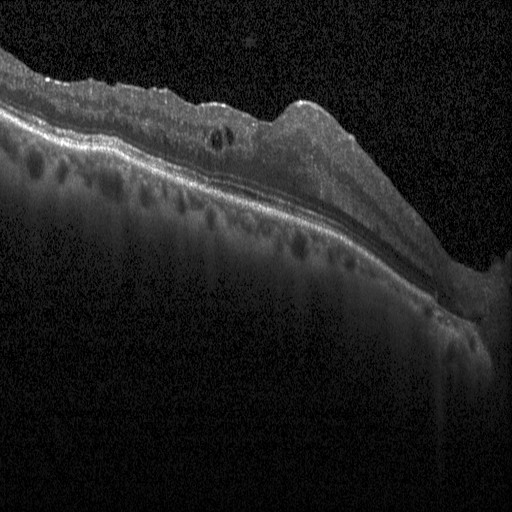
This B-scan demonstrates diabetic macular edema (DME).